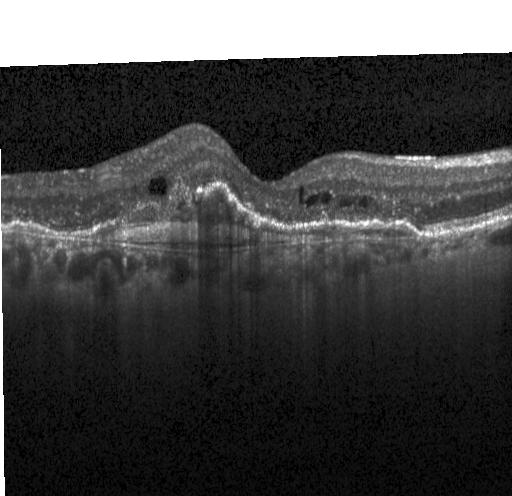

Instrument: Heidelberg Spectralis. Retinal OCT B-scan. Centered on the fovea. Spectral-domain optical coherence tomography.
Impression: a choroidal neovascular membrane.